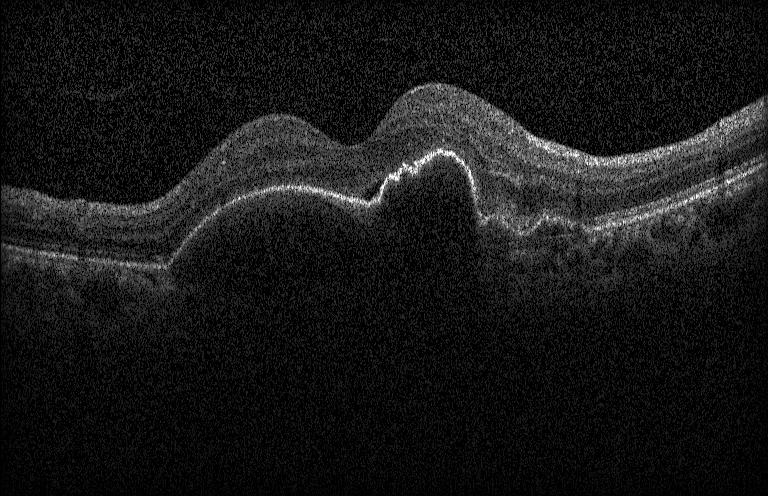 OCT finding: a choroidal neovascular membrane.